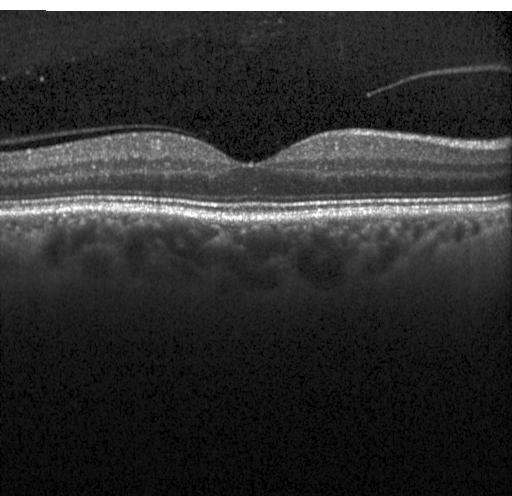 OCT finding: no evidence of choroidal neovascularization, diabetic macular edema, or drusen.